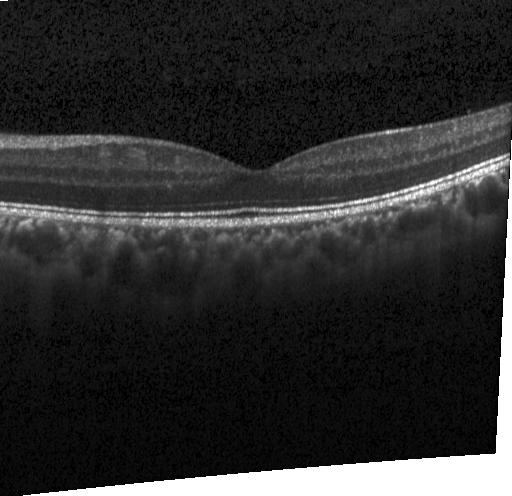

Assessment: no evidence of choroidal neovascularization, diabetic macular edema, or drusen.